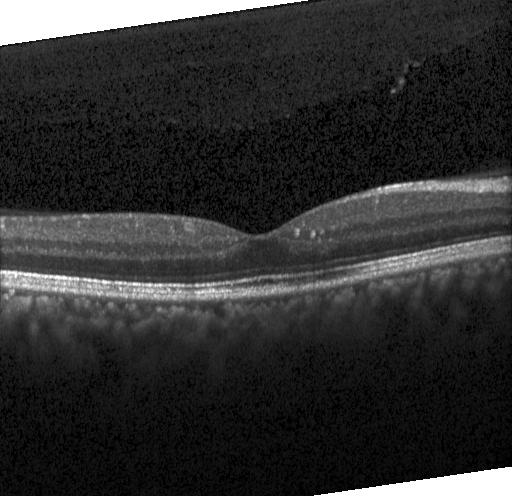 Macular OCT demonstrating neither choroidal neovascularization, diabetic macular edema, nor drusen.